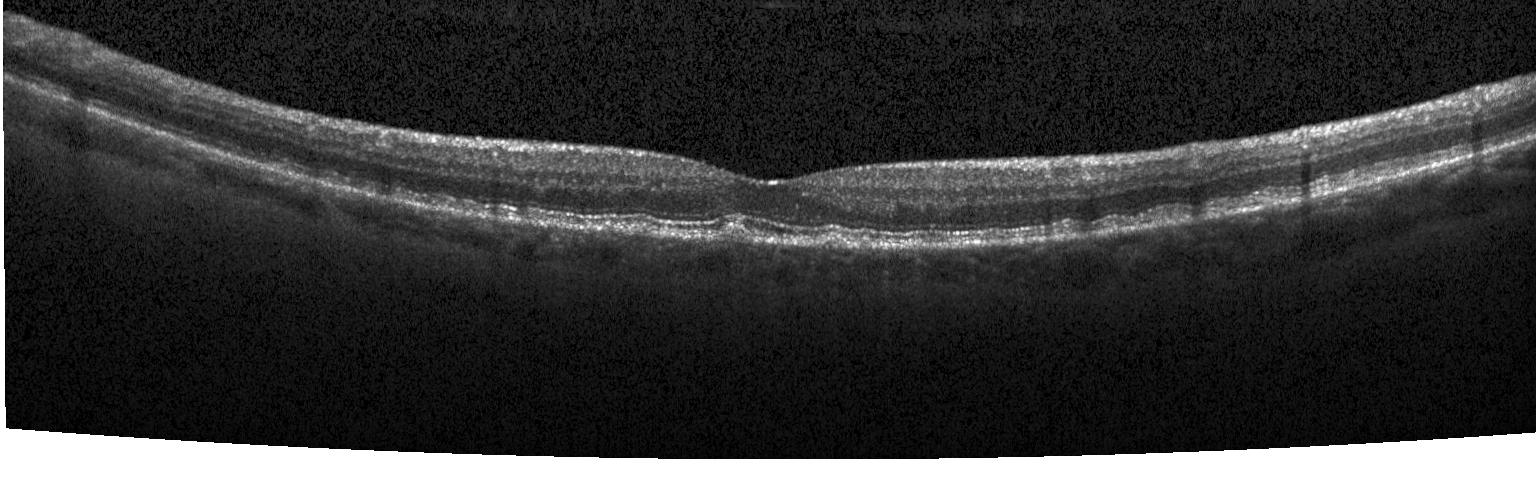 OCT scan showing multiple drusen.